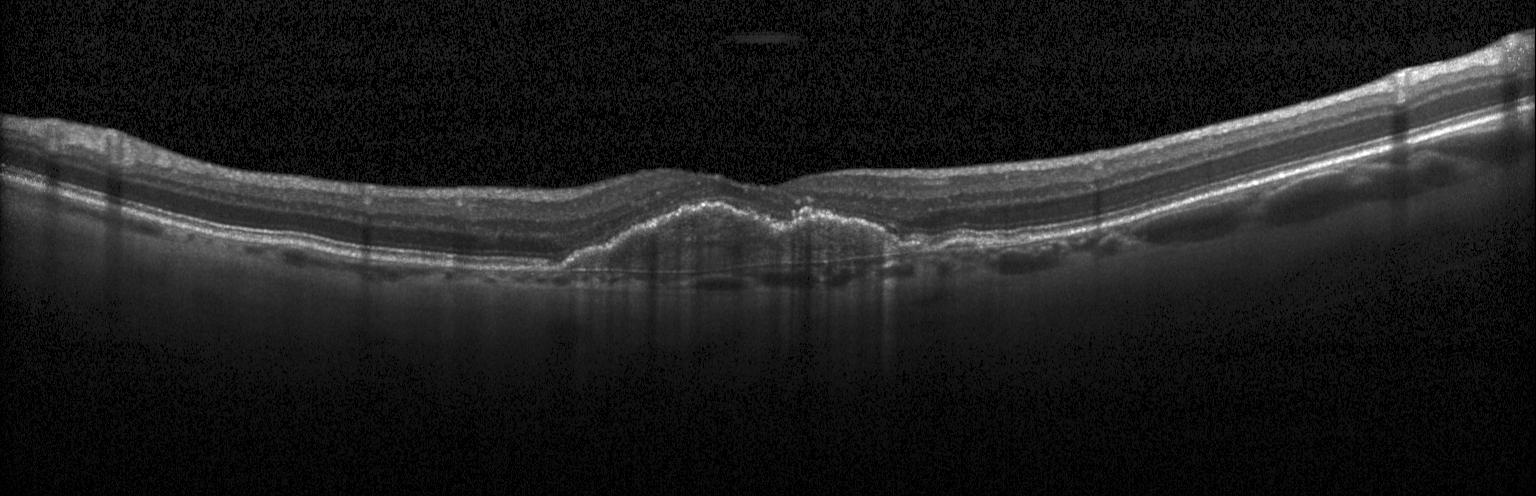
Retinal OCT B-scan. Through the macula
The scan shows a choroidal neovascular membrane.